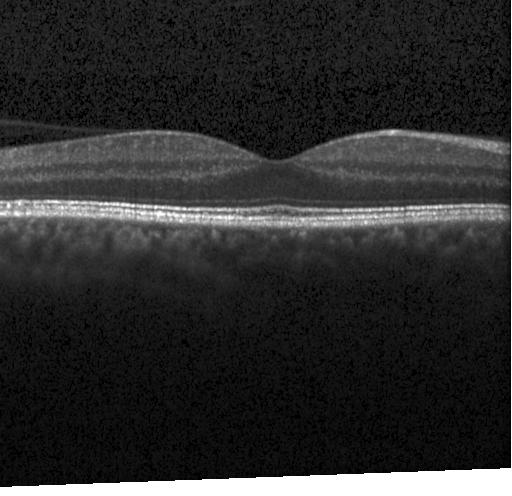 Macular scan · retinal OCT cross-section · spectral-domain OCT. The scan shows no choroidal neovascularization, diabetic macular edema, or drusen.